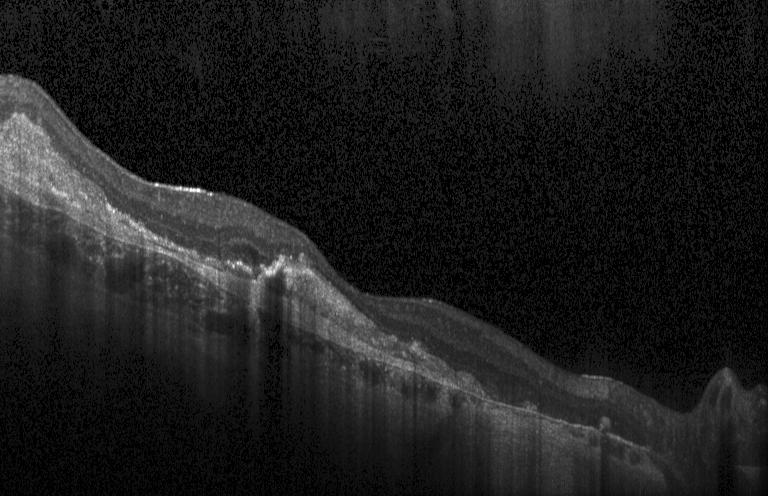 Heidelberg Spectralis OCT system. Retinal OCT cross-section. SD-OCT.
Impression: a choroidal neovascular membrane.